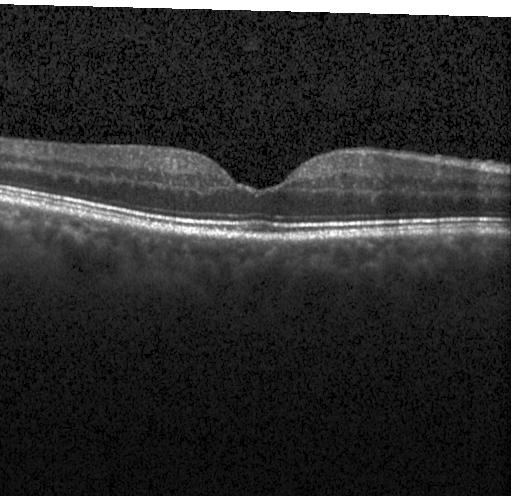 OCT line scan · spectral-domain optical coherence tomography · fovea-centered — OCT finding: no CNV, DME, or drusen.